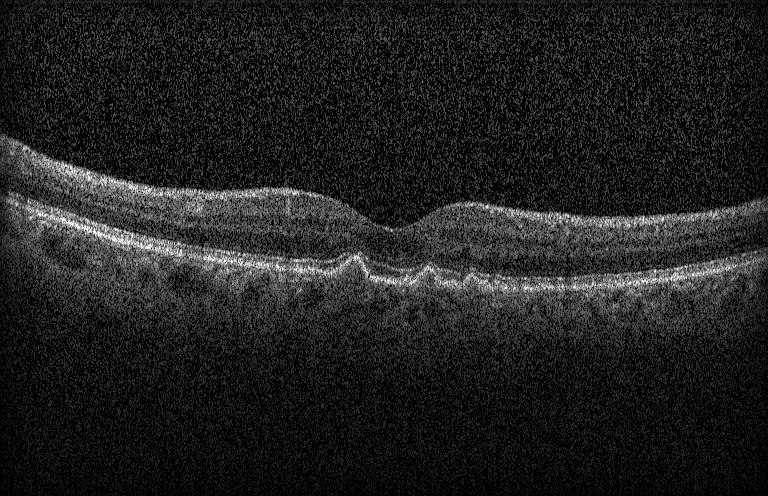 Fovea-centered; OCT B-scan; Heidelberg Spectralis OCT system; spectral-domain OCT
Diagnosis: drusen.